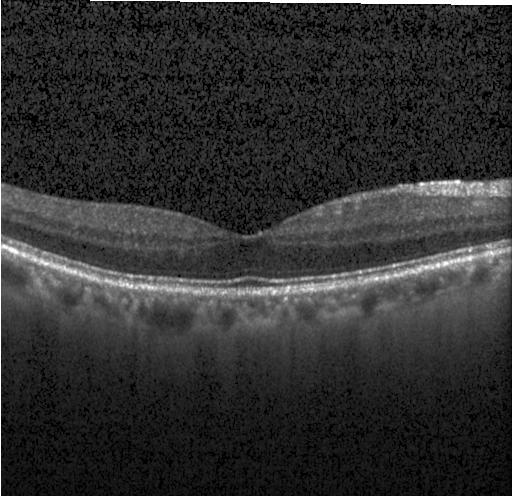 OCT B-scan. Fovea-centered — Impression: no choroidal neovascularization, no diabetic macular edema, and no drusen.